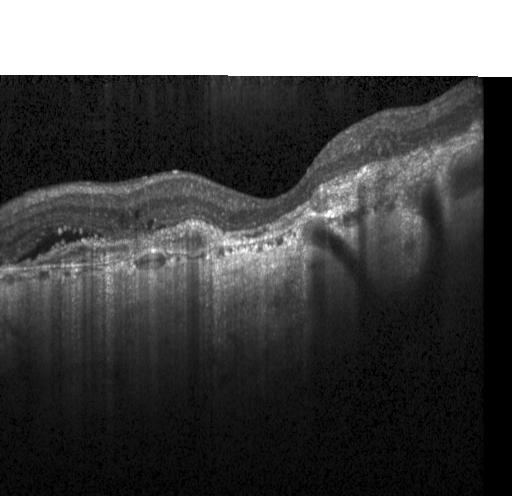

Acquired on a Heidelberg Spectralis, spectral-domain OCT, OCT B-scan.
A choroidal neovascular membrane.